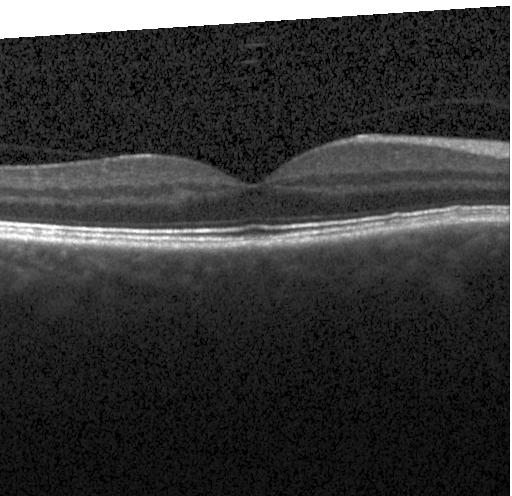

Macular scan, spectral-domain optical coherence tomography, Heidelberg Spectralis, optical coherence tomography scan
Assessment: neither CNV, DME, nor drusen.